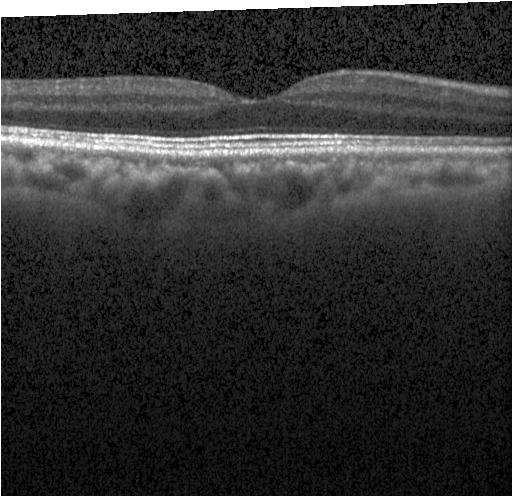 Finding: neither choroidal neovascularization, diabetic macular edema, nor drusen.